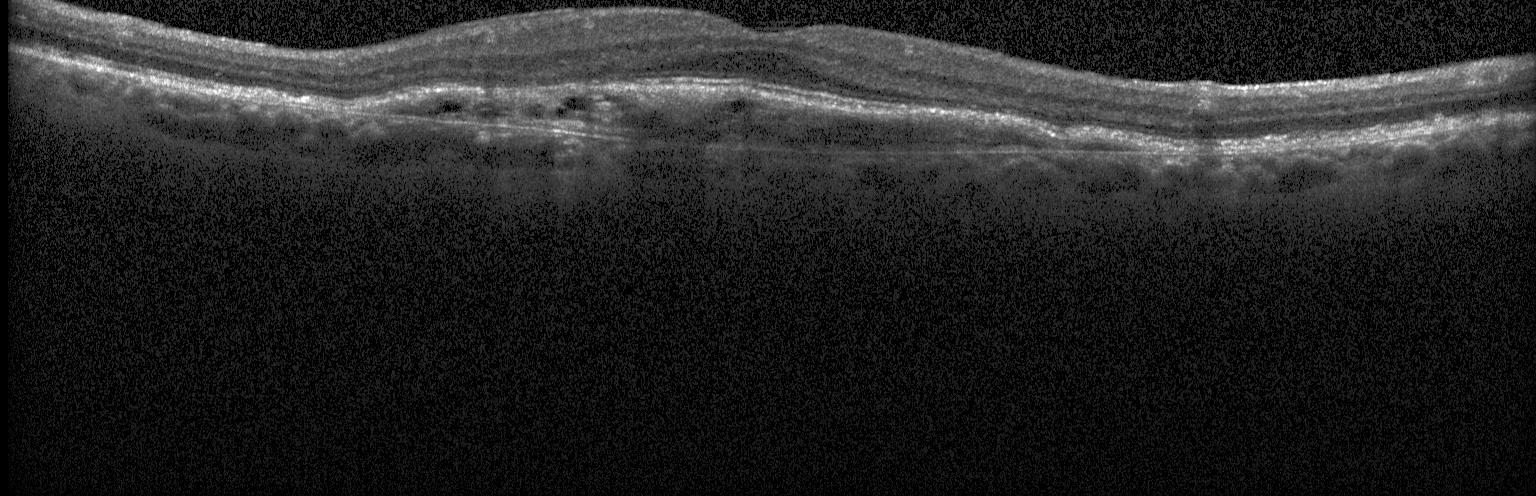

Retinal OCT B-scan. The scan shows CNV.